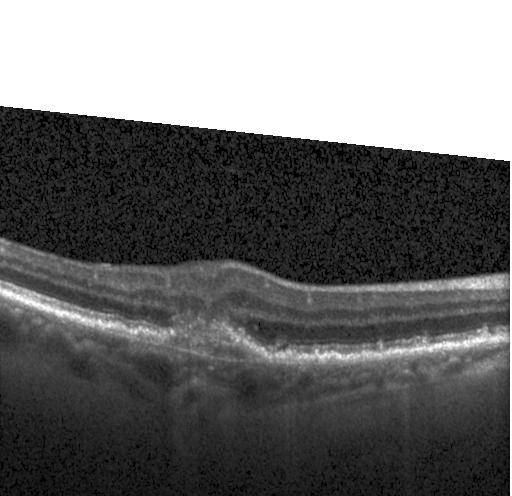
Retinal OCT B-scan; spectral-domain OCT; instrument: Heidelberg Spectralis.
The scan shows a choroidal neovascular membrane.